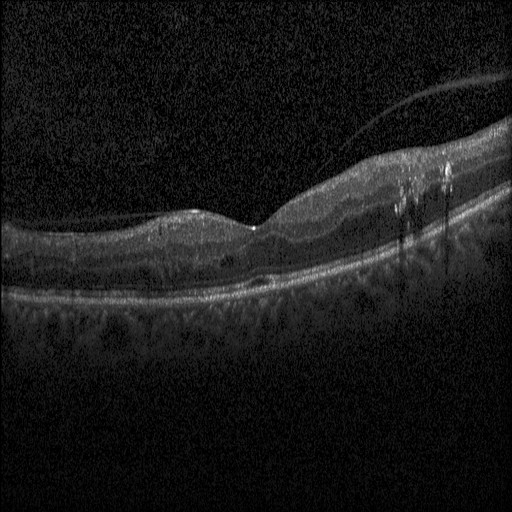

Heidelberg Spectralis OCT system, optical coherence tomography scan, SD-OCT
Diagnosis: diabetic macular edema (DME).